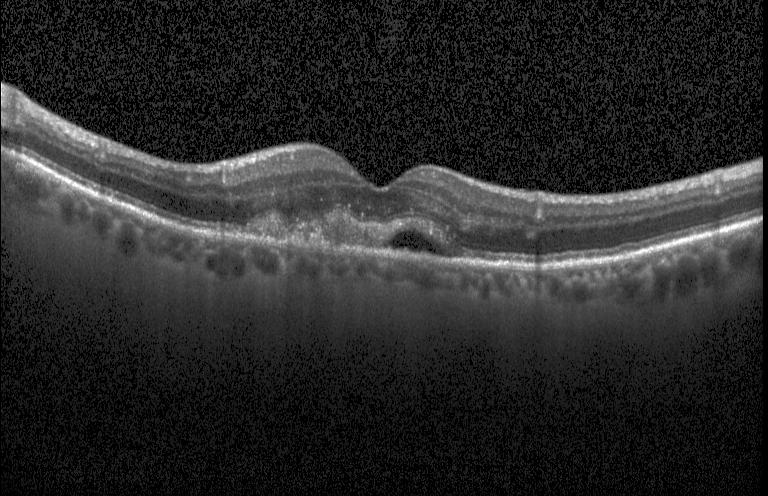
Retinal OCT cross-section
Finding: a choroidal neovascular membrane.